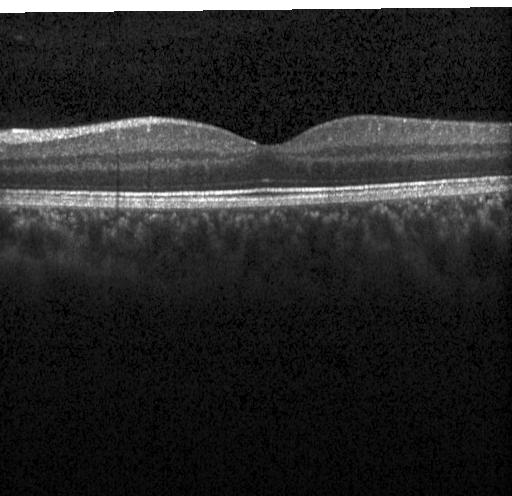
Optical coherence tomography B-scan. SD-OCT. Diagnosis: neither choroidal neovascularization, diabetic macular edema, nor drusen.